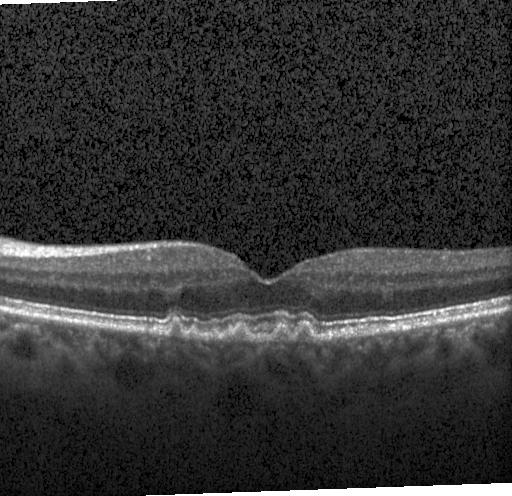 OCT B-scan showing multiple drusen.